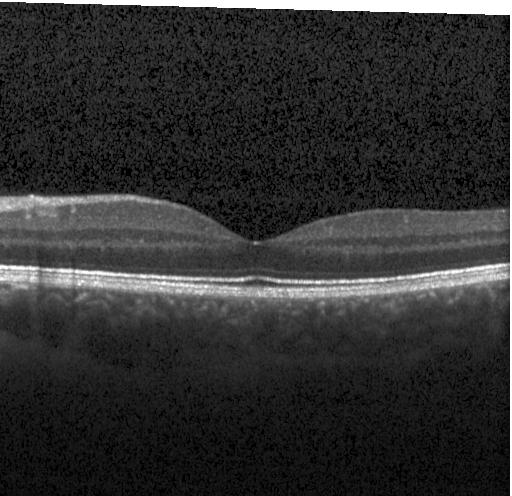

Impression: neither CNV, DME, nor drusen.